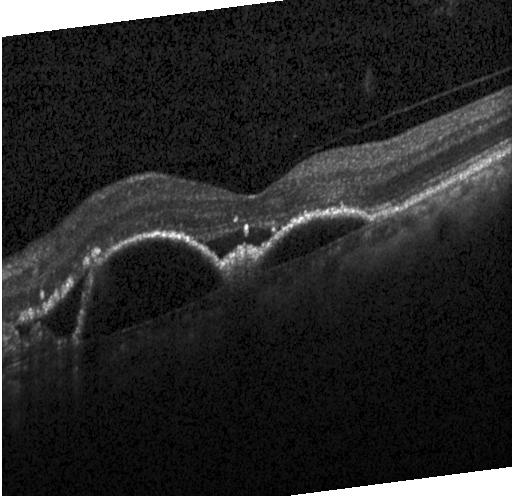
OCT finding: choroidal neovascularization.